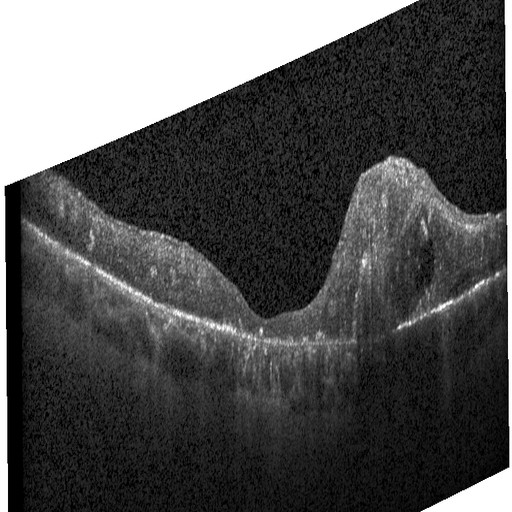 Spectral-domain OCT; instrument: Heidelberg Spectralis; optical coherence tomography B-scan — Diabetic macular edema.